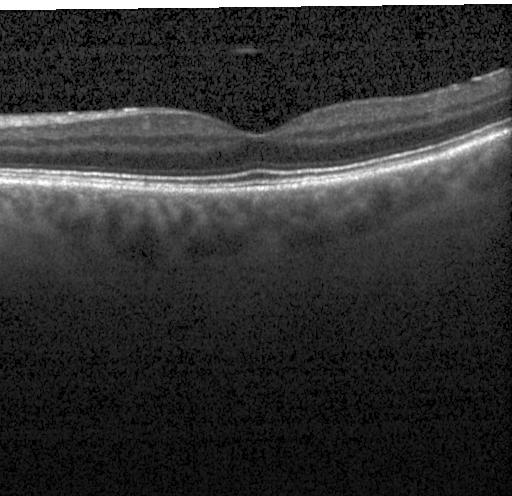 OCT B-scan; instrument: Heidelberg Spectralis; centered on the fovea
Finding: neither choroidal neovascularization, diabetic macular edema, nor drusen.